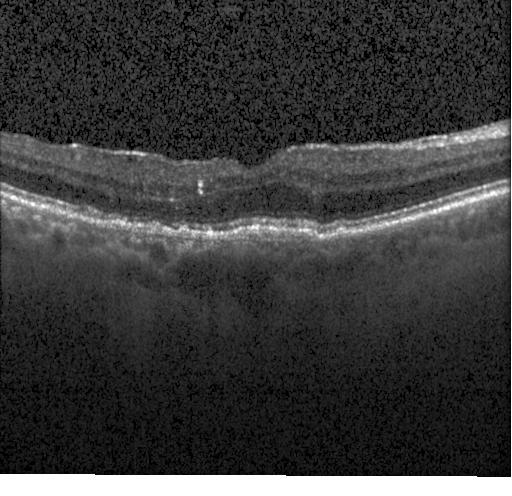 Dx: a choroidal neovascular membrane.